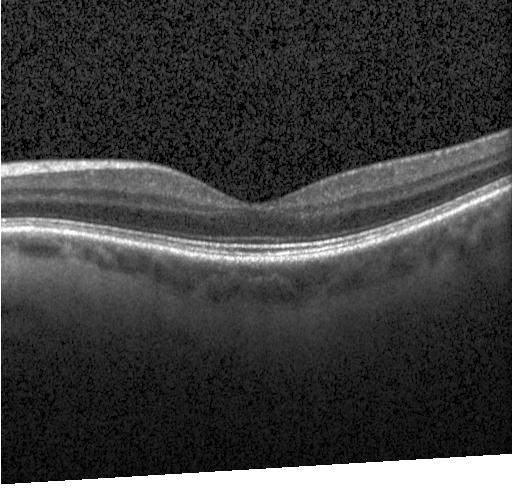 Finding: no evidence of choroidal neovascularization, diabetic macular edema, or drusen.